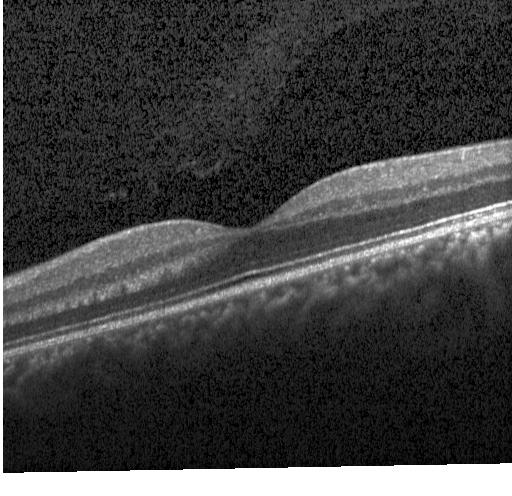 OCT line scan. Diagnosis: no evidence of choroidal neovascularization, diabetic macular edema, or drusen.